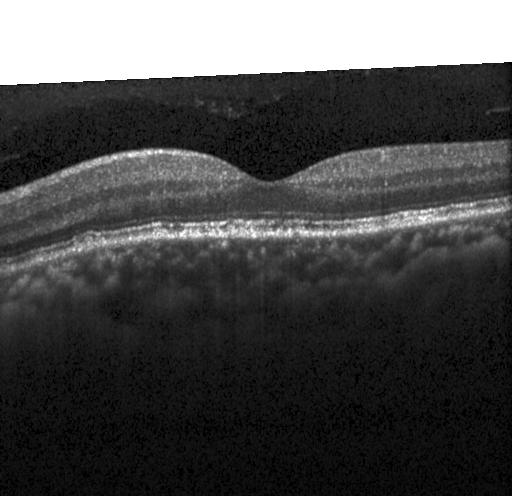 Macular OCT: sub-RPE drusenoid deposits.